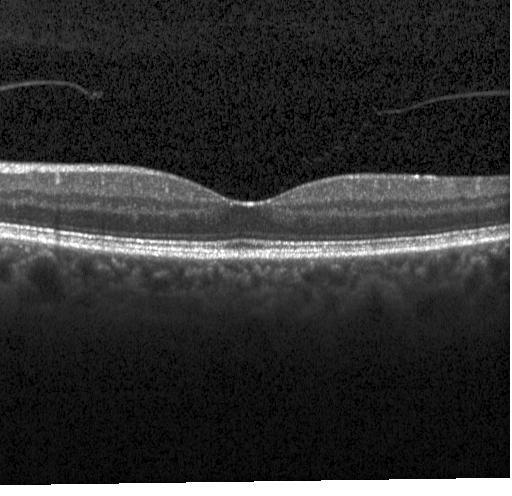 Optical coherence tomography B-scan.
This B-scan demonstrates neither CNV, DME, nor drusen.